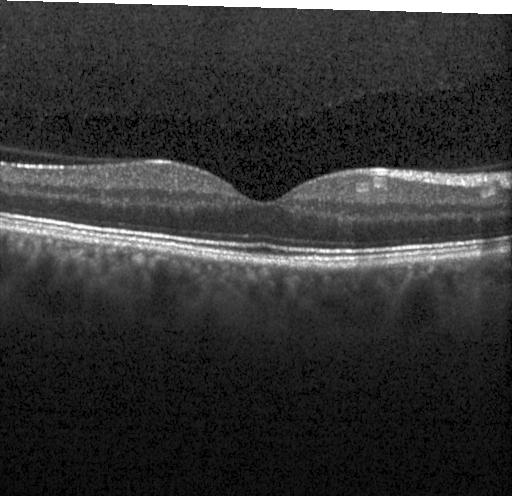 Optical coherence tomography B-scan — Macular OCT: no choroidal neovascularization, diabetic macular edema, or drusen.